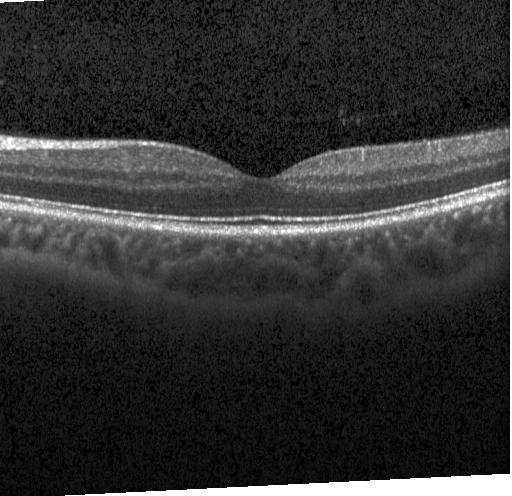 OCT line scan. Macular scan
Assessment: no CNV, no DME, and no drusen.